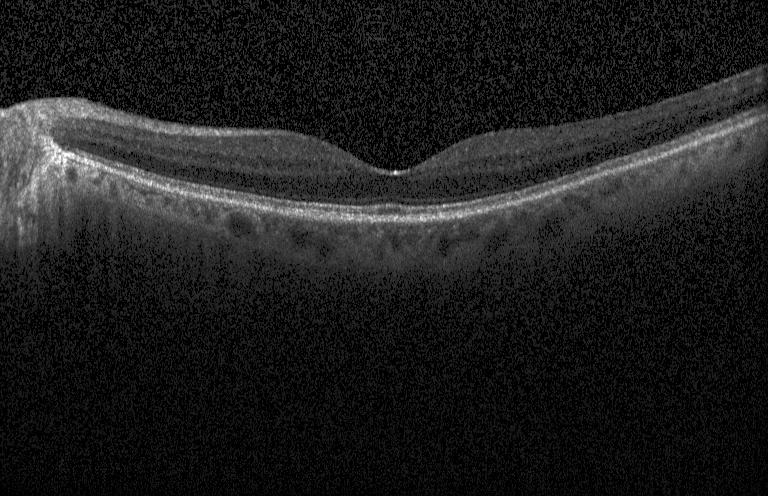
Optical coherence tomography B-scan; centered on the fovea; spectral-domain optical coherence tomography; instrument: Heidelberg Spectralis.
OCT finding: no evidence of choroidal neovascularization, diabetic macular edema, or drusen.